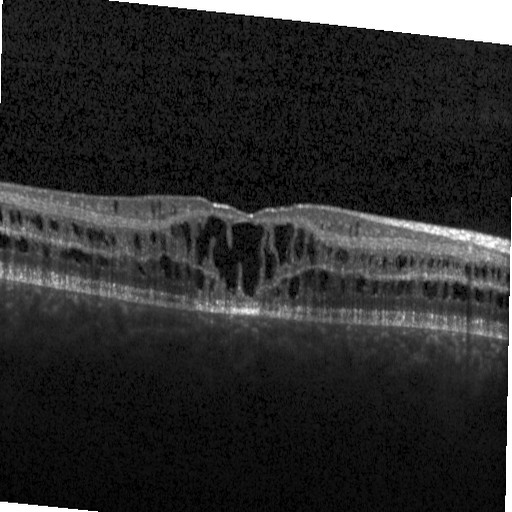 OCT B-scan — Impression: diabetic macular edema (DME).